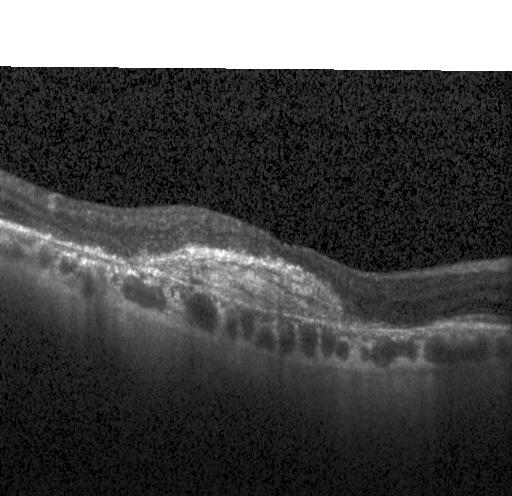 Retinal OCT B-scan · acquired on a Heidelberg Spectralis · spectral-domain OCT · centered on the fovea. Choroidal neovascularization.